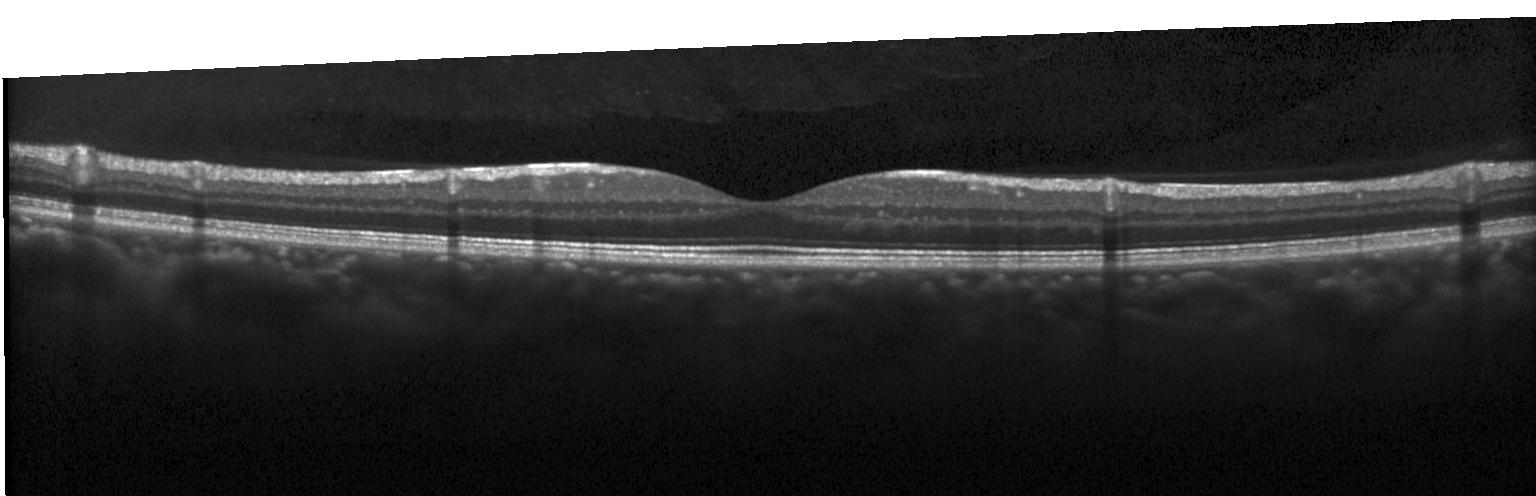
OCT line scan
Impression: neither choroidal neovascularization, diabetic macular edema, nor drusen.